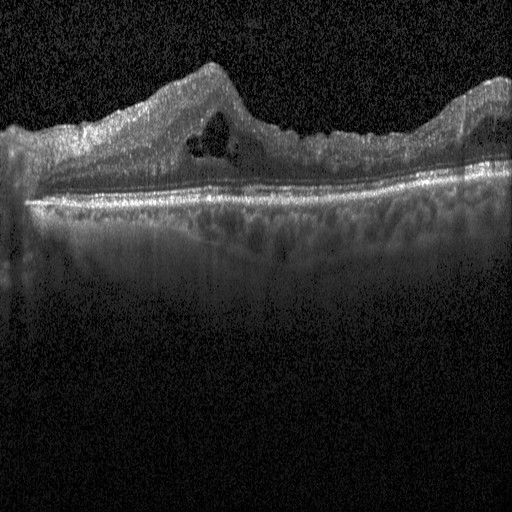
Dx: diabetic macular edema.